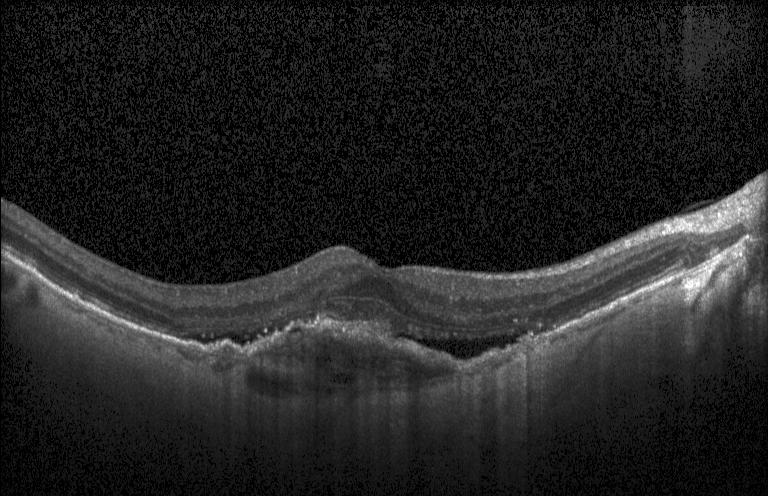

Dx: choroidal neovascularization.